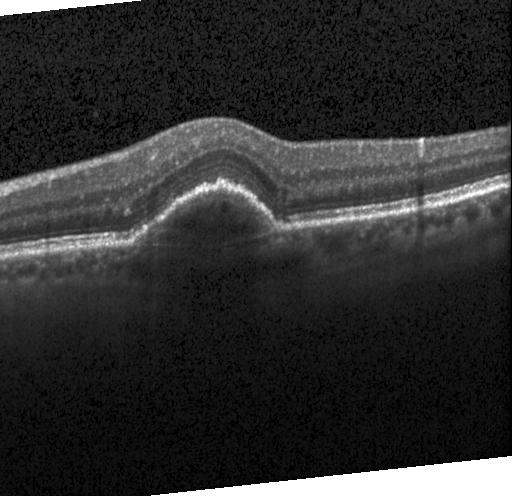 Optical coherence tomography B-scan. Through the macula. Heidelberg Spectralis OCT system.
A choroidal neovascular membrane.